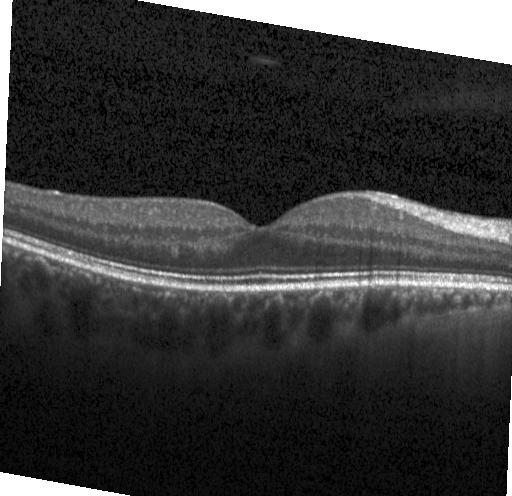
Optical coherence tomography scan.
This B-scan demonstrates no evidence of CNV, DME, or drusen.